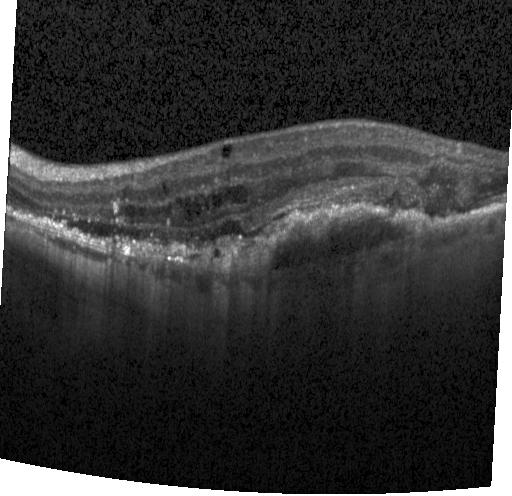 OCT line scan; spectral-domain OCT; Heidelberg Spectralis OCT system; fovea-centered
Finding: a choroidal neovascular membrane.